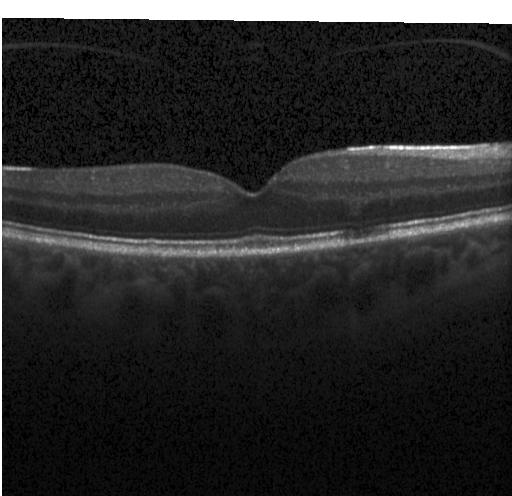 Acquired on a Heidelberg Spectralis. Retinal OCT cross-section. SD-OCT.
The scan shows neither choroidal neovascularization, diabetic macular edema, nor drusen.